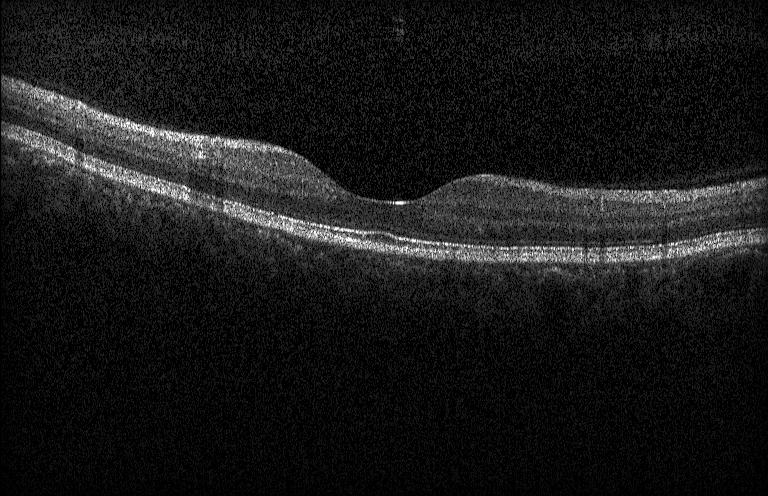

Optical coherence tomography scan. Impression: no choroidal neovascularization, no diabetic macular edema, and no drusen.